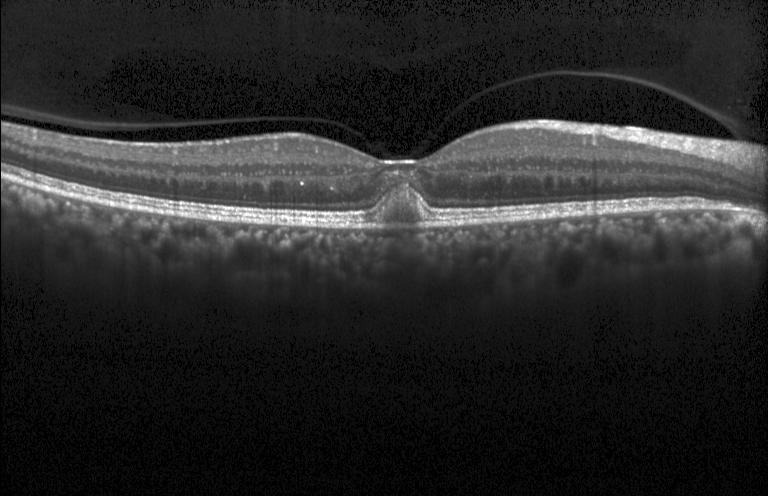

Dx: CNV.